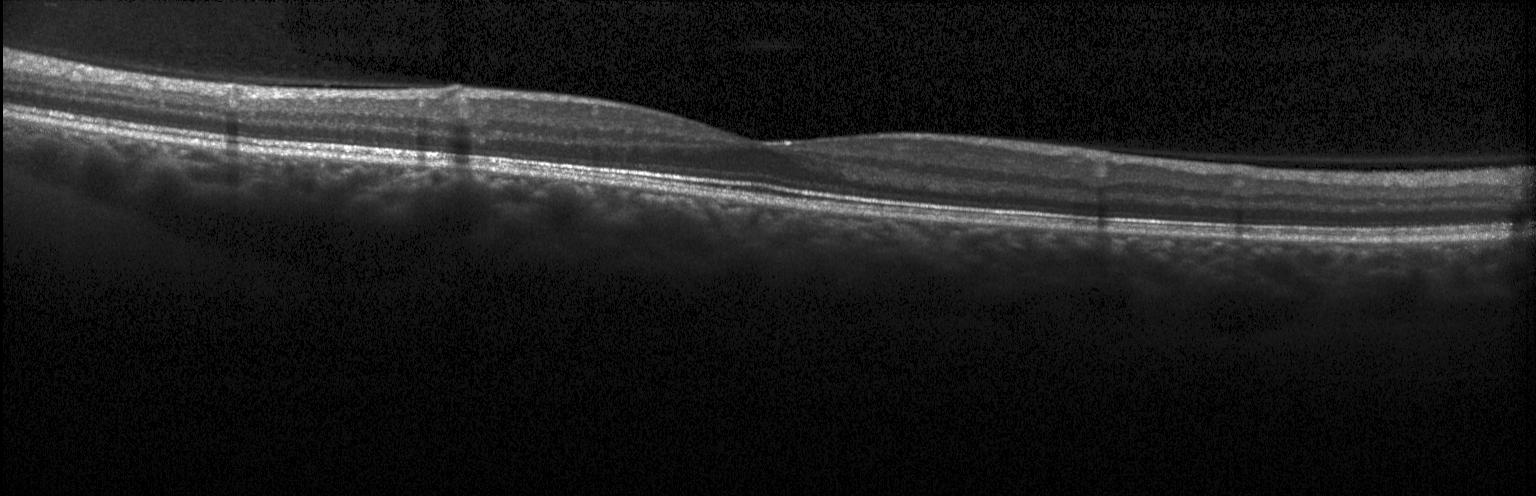
Macular OCT demonstrating neither CNV, DME, nor drusen.